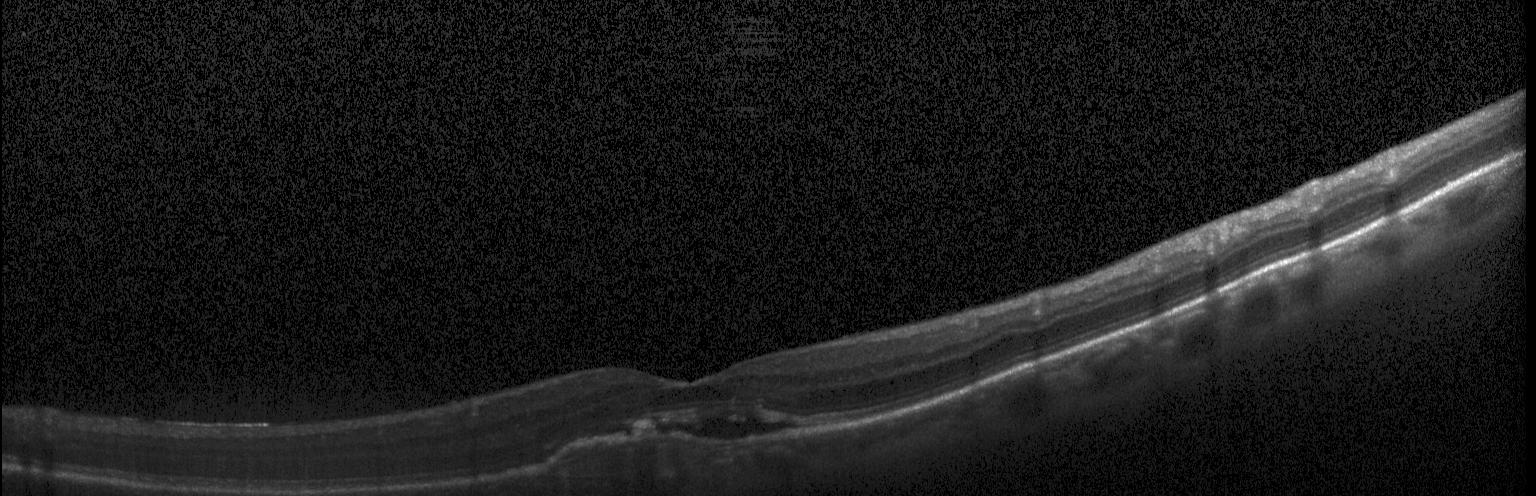

Retinal OCT B-scan; Heidelberg Spectralis OCT system; spectral-domain optical coherence tomography
The scan shows CNV.